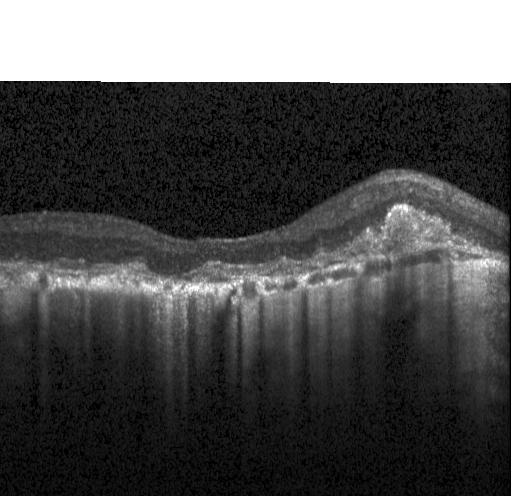
Optical coherence tomography scan · spectral-domain optical coherence tomography · acquired on a Heidelberg Spectralis · macular scan. Macular OCT: a choroidal neovascular membrane.